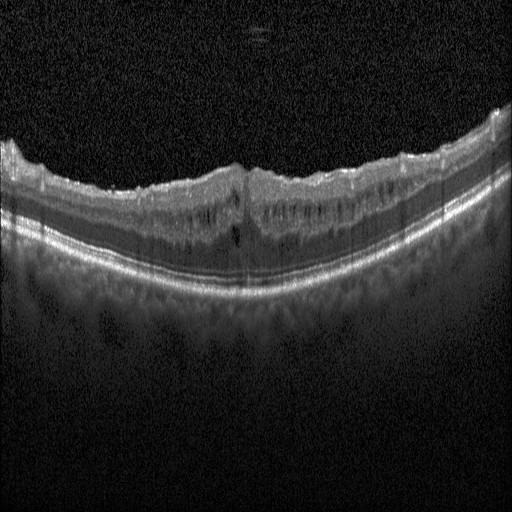 Diabetic macular edema (DME).